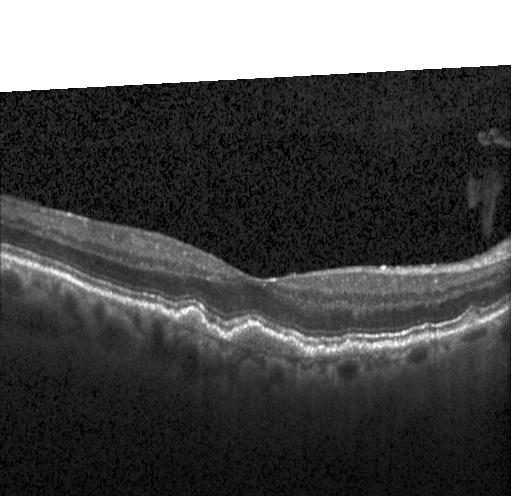
SD-OCT · centered on the fovea · optical coherence tomography B-scan
The scan shows a choroidal neovascular membrane.